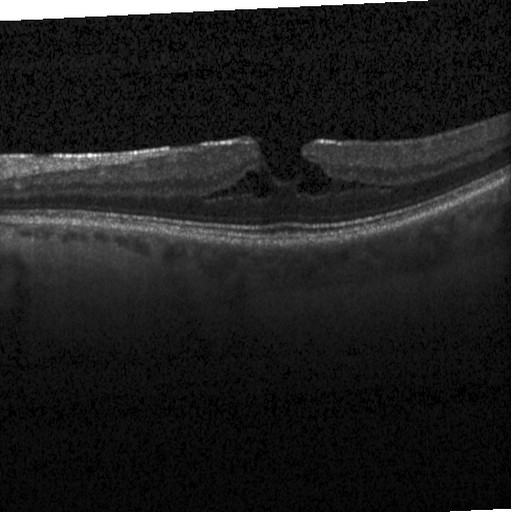
Impression: DME.